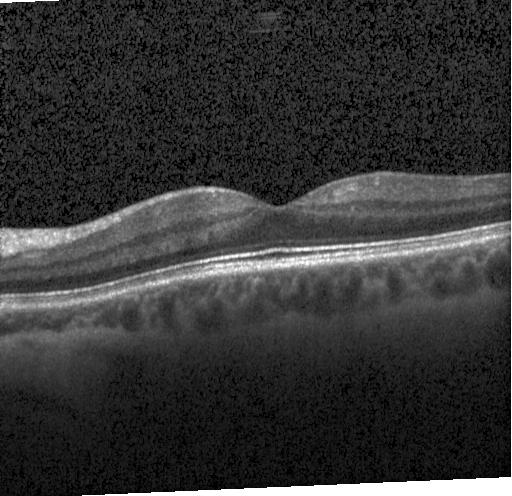
Neither choroidal neovascularization, diabetic macular edema, nor drusen.